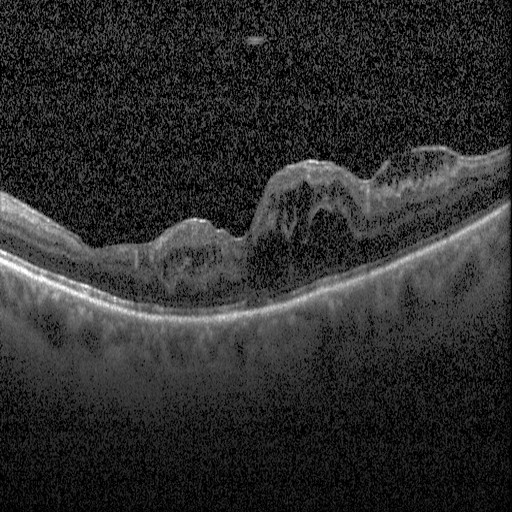
Finding: diabetic macular edema (DME).